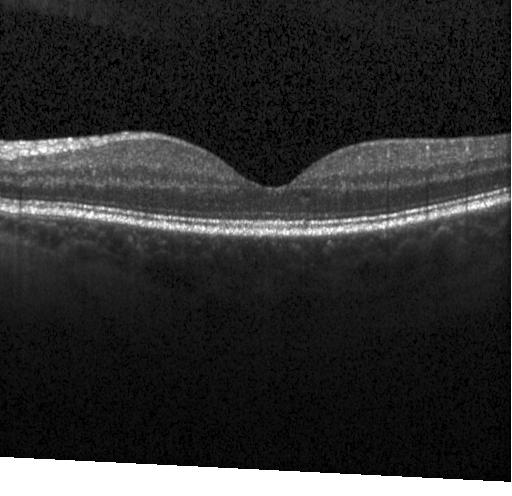 Retinal OCT cross-section
Assessment: no evidence of choroidal neovascularization, diabetic macular edema, or drusen.